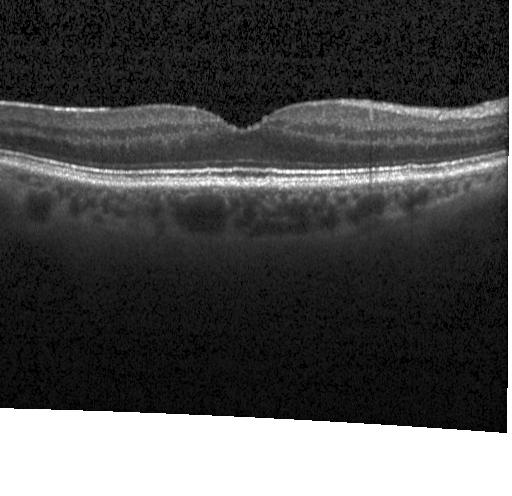

Finding: no CNV, DME, or drusen.